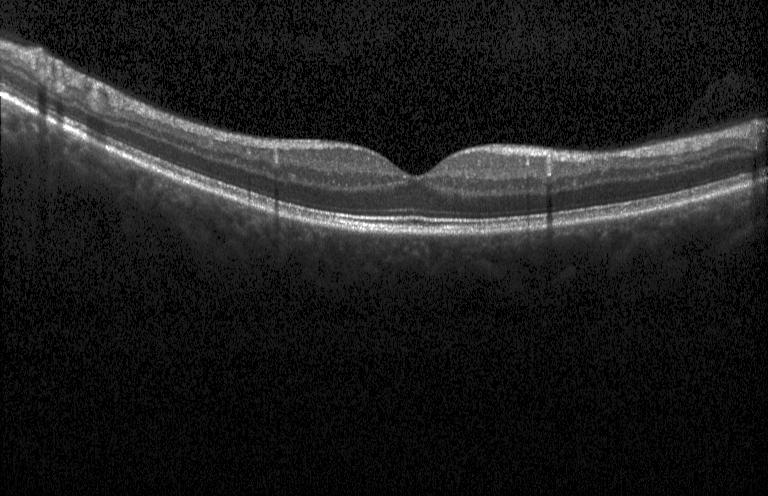

Retinal OCT cross-section showing no choroidal neovascularization, no diabetic macular edema, and no drusen.